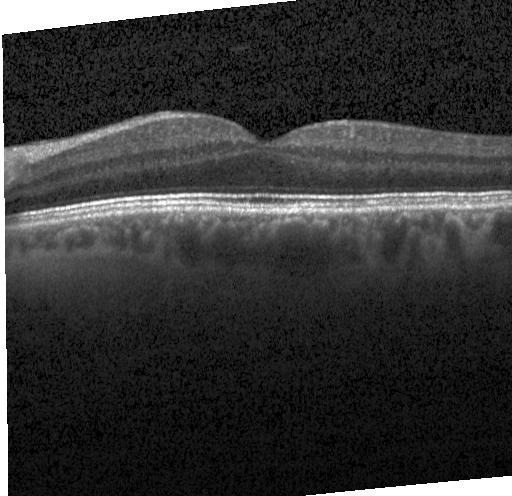

Spectral-domain OCT B-scan: neither CNV, DME, nor drusen.